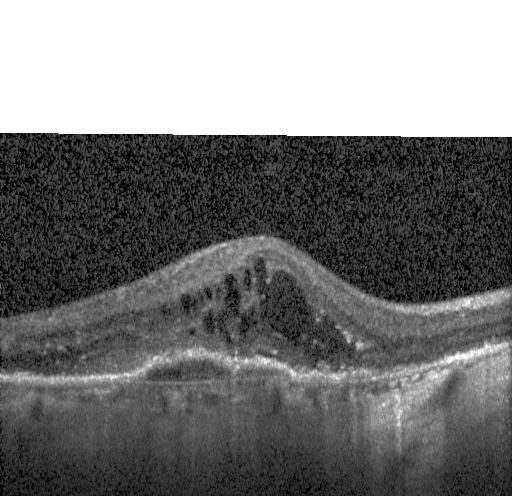
Retinal OCT cross-section showing CNV.